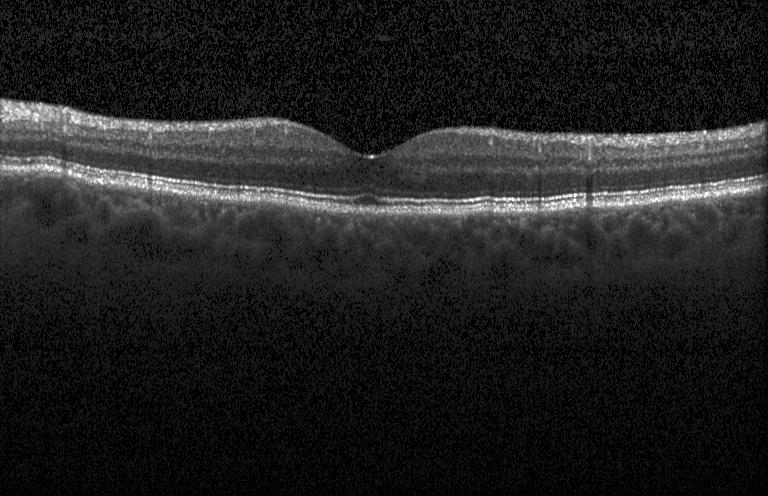
Spectral-domain OCT B-scan: no choroidal neovascularization, no diabetic macular edema, and no drusen.